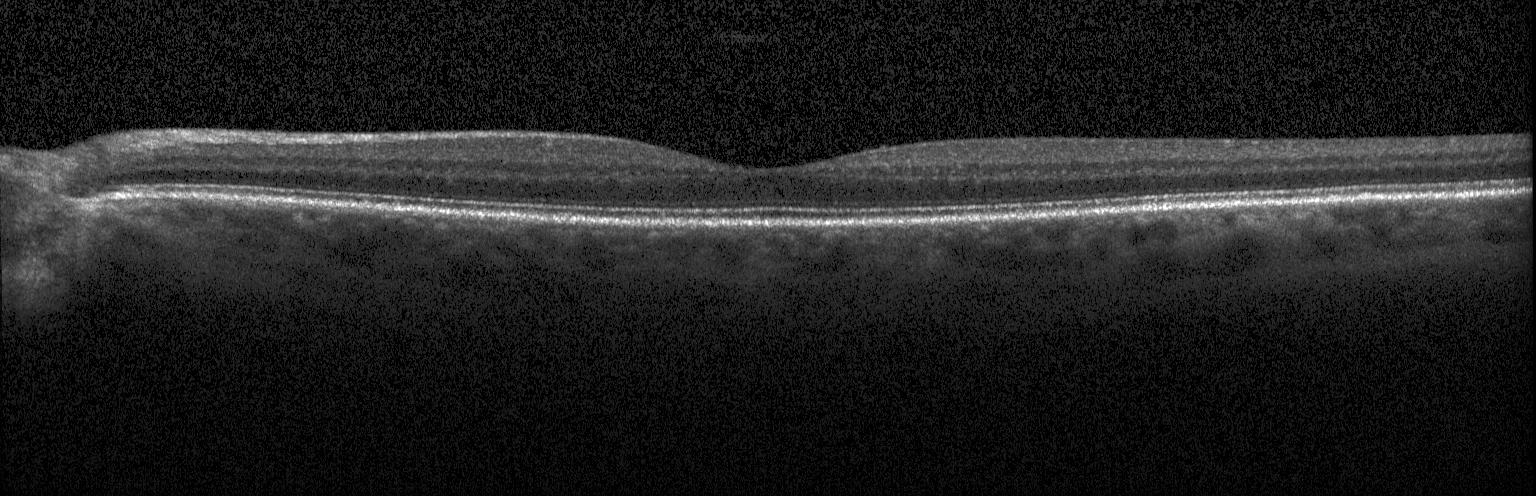 Fovea-centered, Heidelberg Spectralis, OCT B-scan — The scan shows no choroidal neovascularization, diabetic macular edema, or drusen.